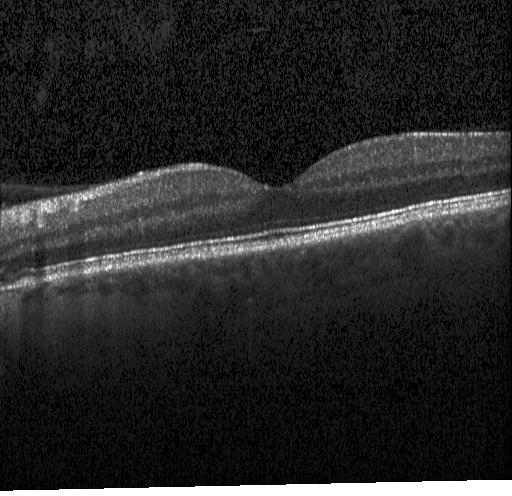 OCT line scan
Assessment: no evidence of CNV, DME, or drusen.